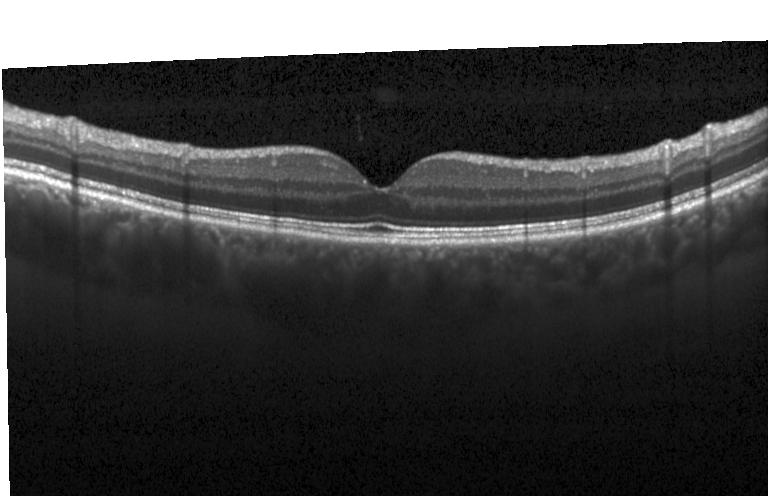
SD-OCT, retinal OCT cross-section.
Impression: no evidence of choroidal neovascularization, diabetic macular edema, or drusen.